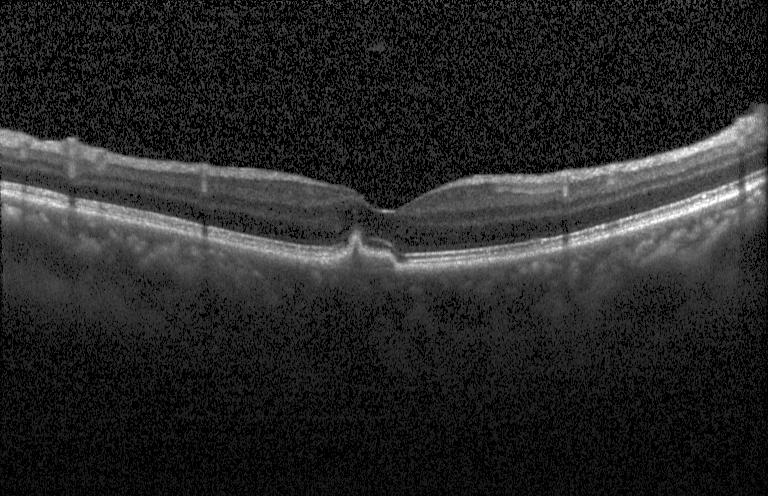

Fovea-centered; spectral-domain OCT; Heidelberg Spectralis; OCT line scan.
Multiple drusen.